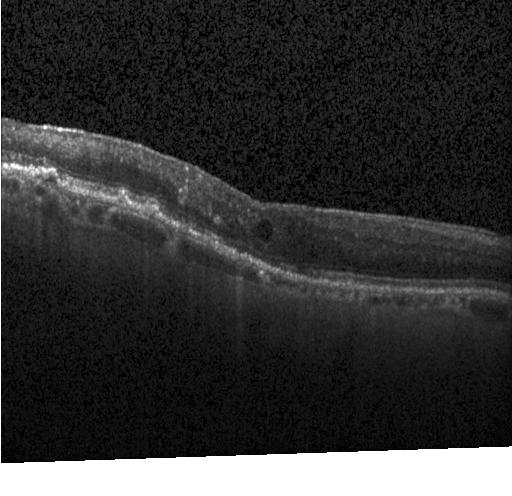

Optical coherence tomography scan
OCT finding: CNV.